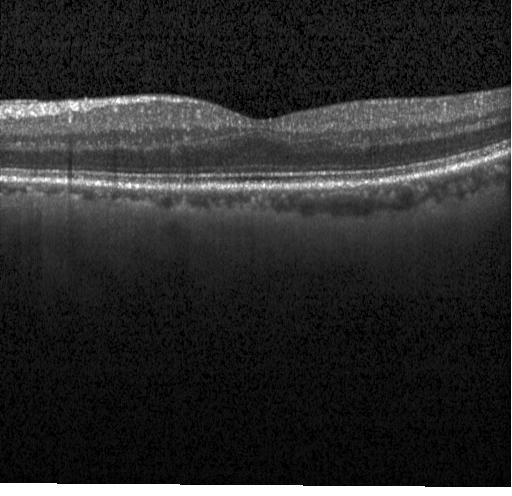
Instrument: Heidelberg Spectralis · retinal OCT cross-section.
Finding: no choroidal neovascularization, diabetic macular edema, or drusen.